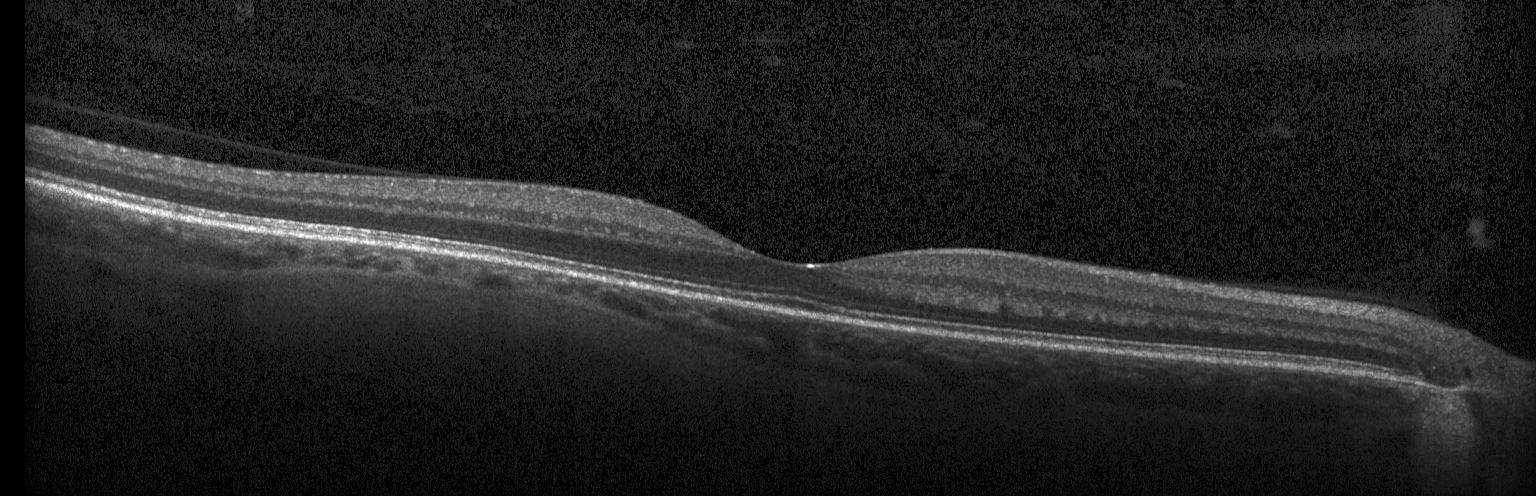 Macular OCT demonstrating no choroidal neovascularization, no diabetic macular edema, and no drusen.